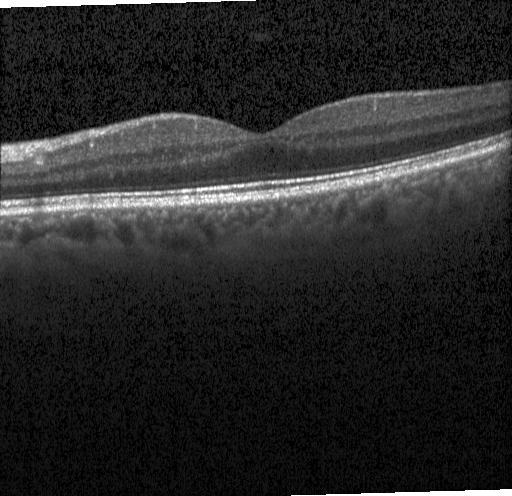 Dx: no choroidal neovascularization, no diabetic macular edema, and no drusen.